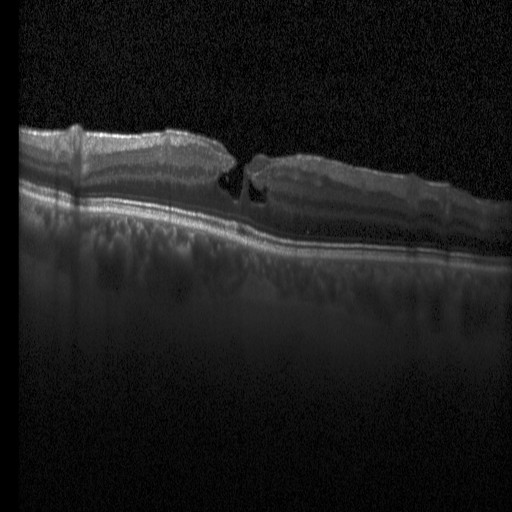 Finding: DME.